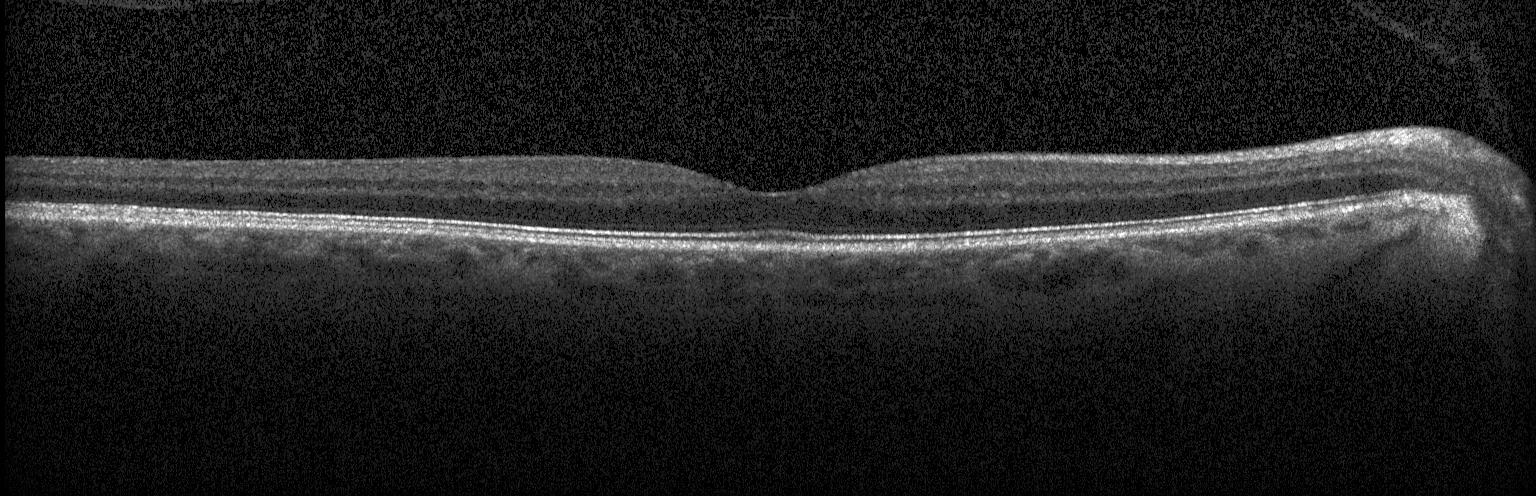
Horizontal scan through the fovea, spectral-domain optical coherence tomography, instrument: Heidelberg Spectralis, OCT line scan — Macular OCT: no evidence of CNV, DME, or drusen.